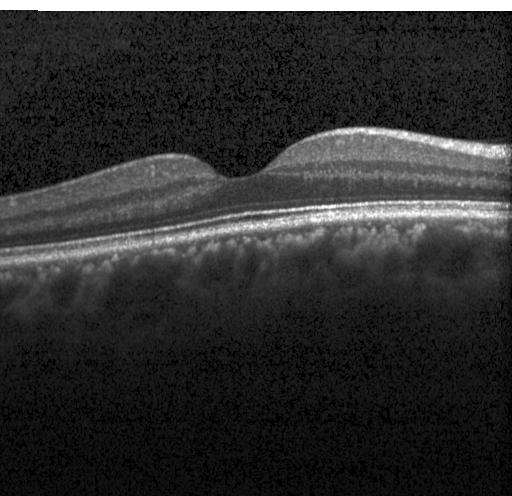 Spectral-domain OCT, retinal OCT B-scan, Heidelberg Spectralis, horizontal scan through the fovea. Assessment: no choroidal neovascularization, no diabetic macular edema, and no drusen.